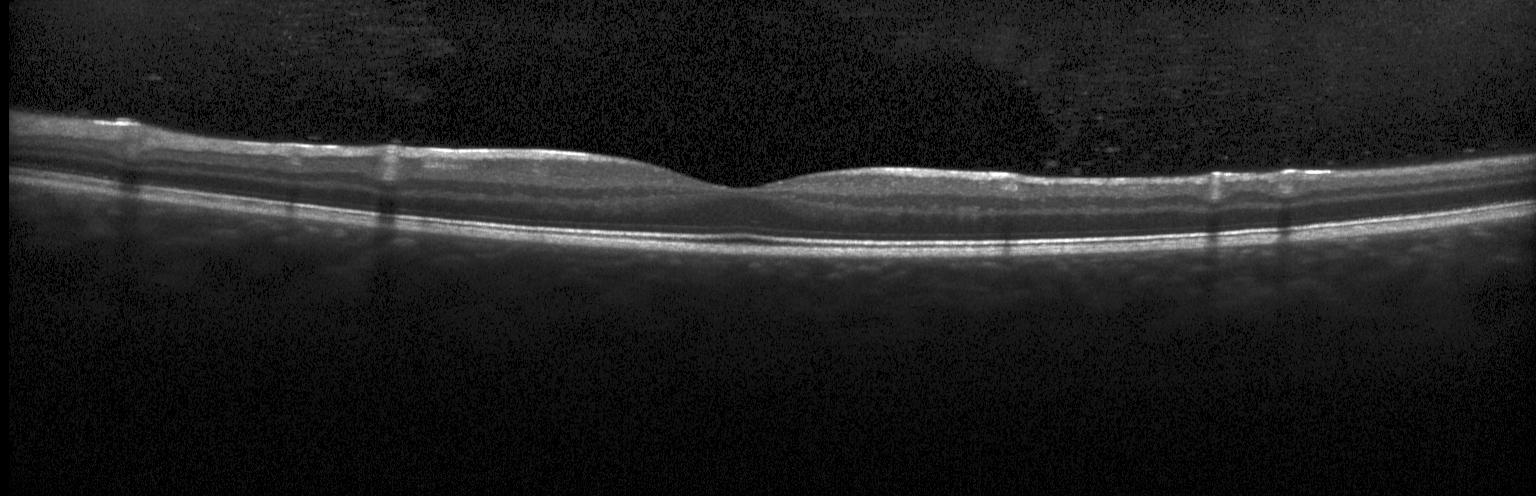
Retinal OCT cross-section.
This B-scan demonstrates no choroidal neovascularization, diabetic macular edema, or drusen.